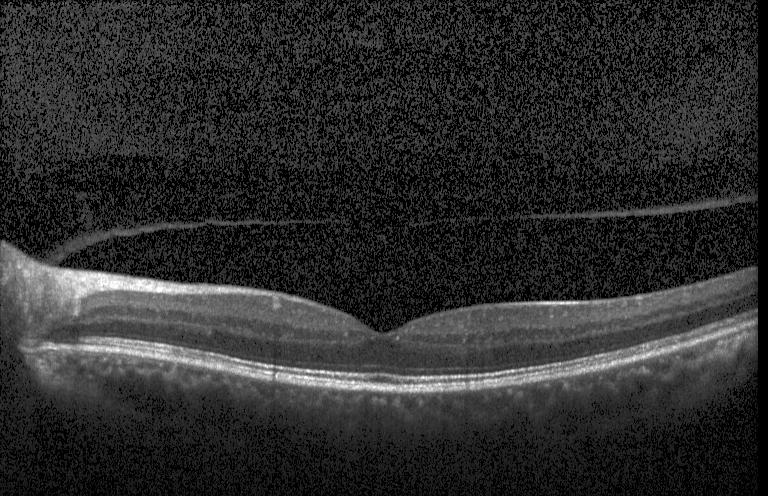

No choroidal neovascularization, no diabetic macular edema, and no drusen.